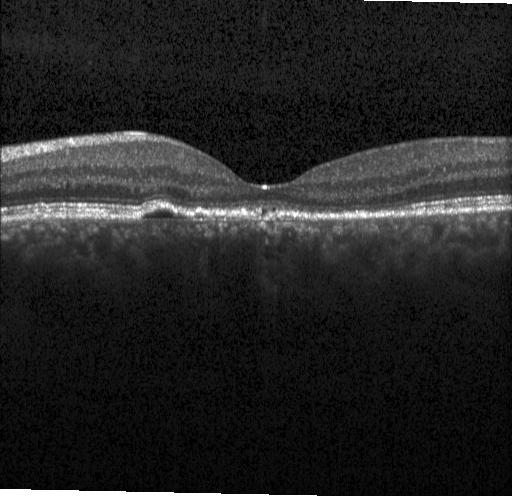
OCT line scan. Impression: a choroidal neovascular membrane.